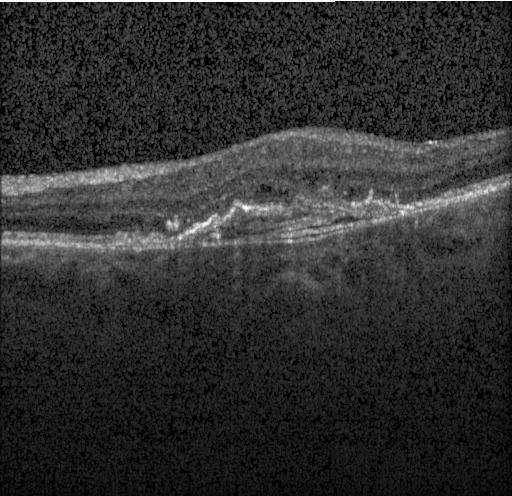

The scan shows choroidal neovascularization (CNV).